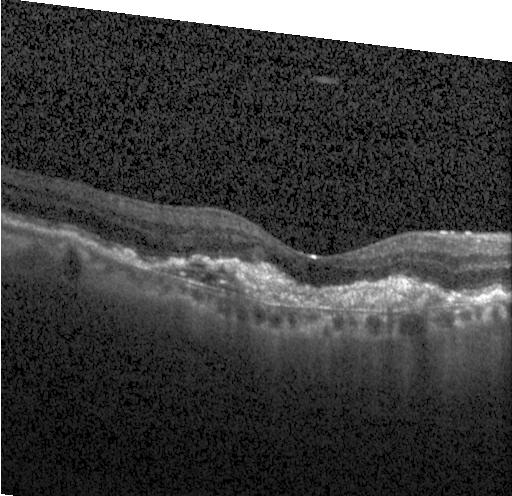
Macular scan. Heidelberg Spectralis. OCT B-scan.
Macular OCT: choroidal neovascularization (CNV).